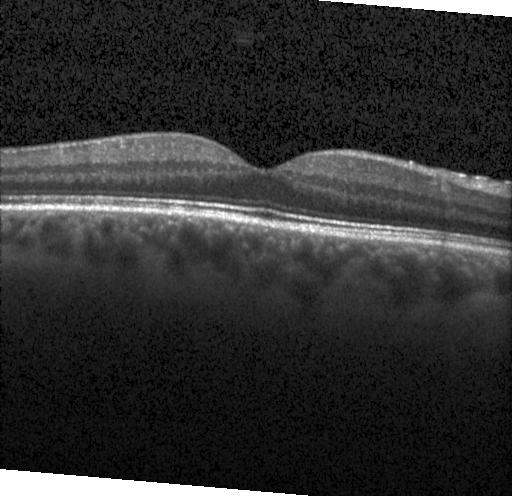

Optical coherence tomography B-scan.
OCT finding: no choroidal neovascularization, diabetic macular edema, or drusen.